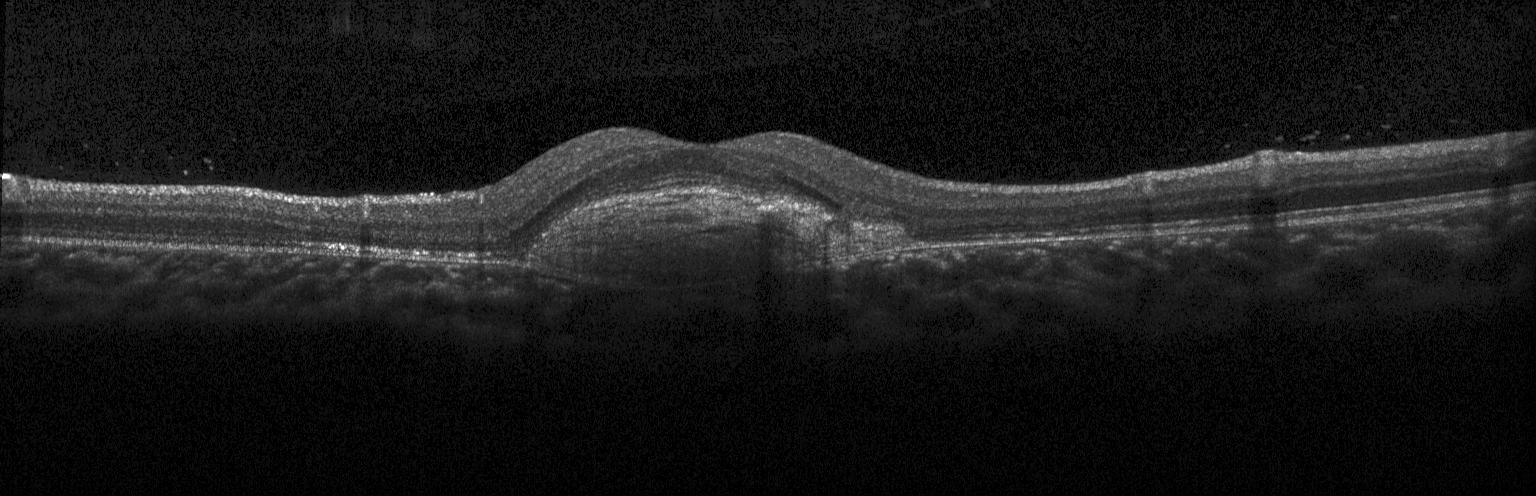 Diagnosis: a choroidal neovascular membrane.